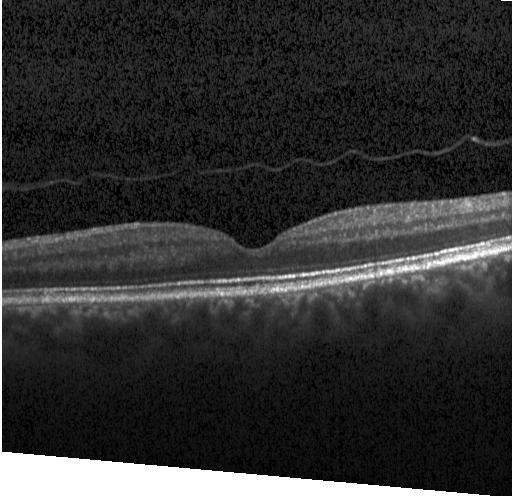

Optical coherence tomography scan
Dx: neither CNV, DME, nor drusen.